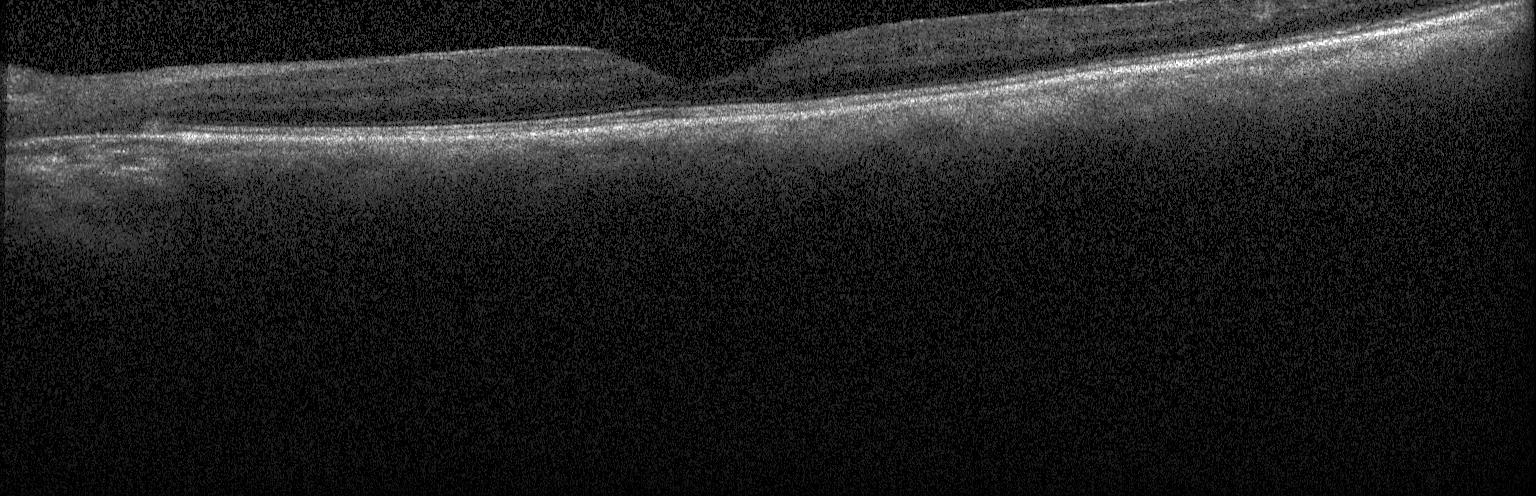
OCT line scan. Spectral-domain optical coherence tomography. Heidelberg Spectralis. Assessment: no CNV, no DME, and no drusen.